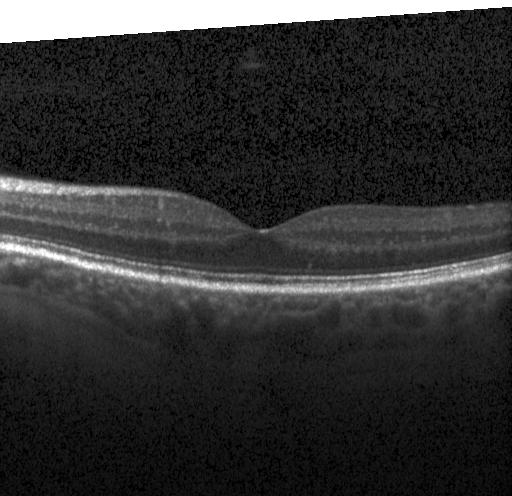 Centered on the fovea; retinal OCT B-scan. Impression: no CNV, no DME, and no drusen.